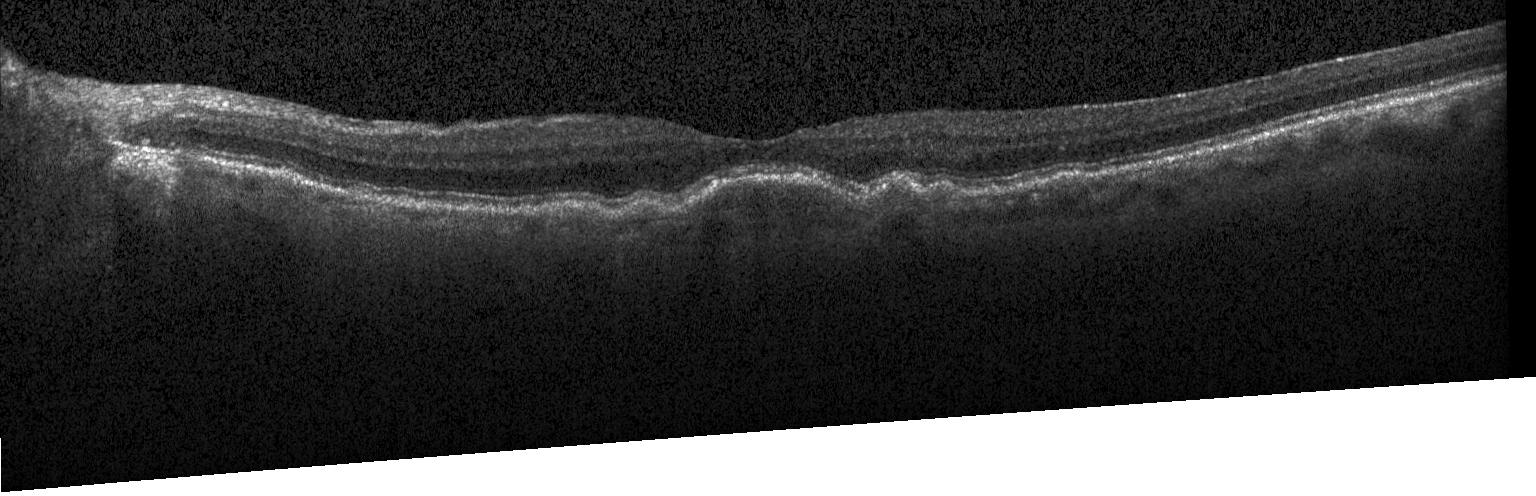 Through the macula, OCT B-scan, Heidelberg Spectralis OCT system, SD-OCT
Macular OCT: choroidal neovascularization.